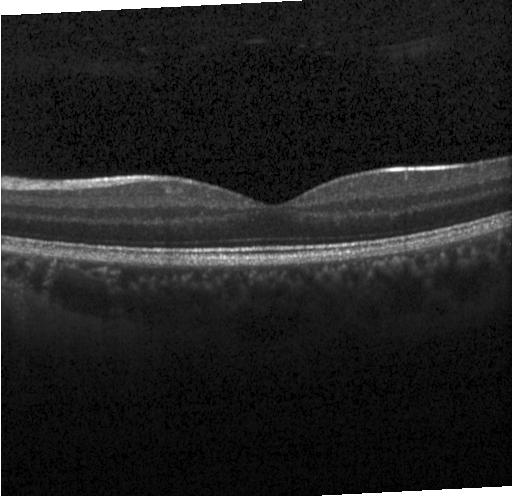
No choroidal neovascularization, no diabetic macular edema, and no drusen.